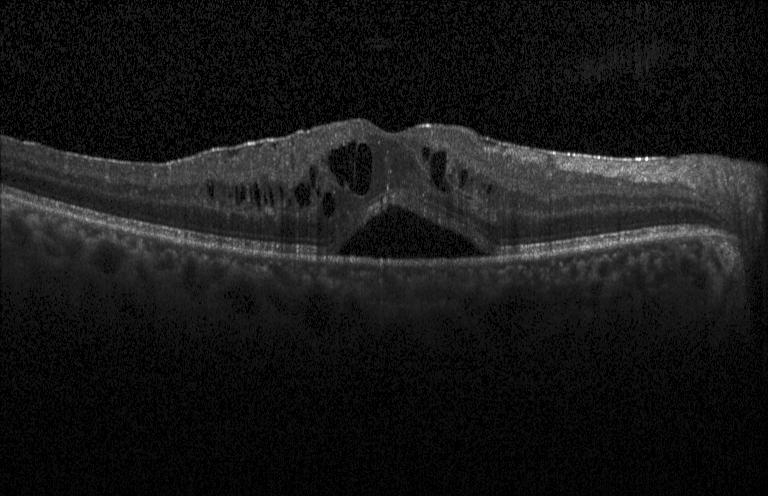

OCT B-scan
Diabetic macular edema.